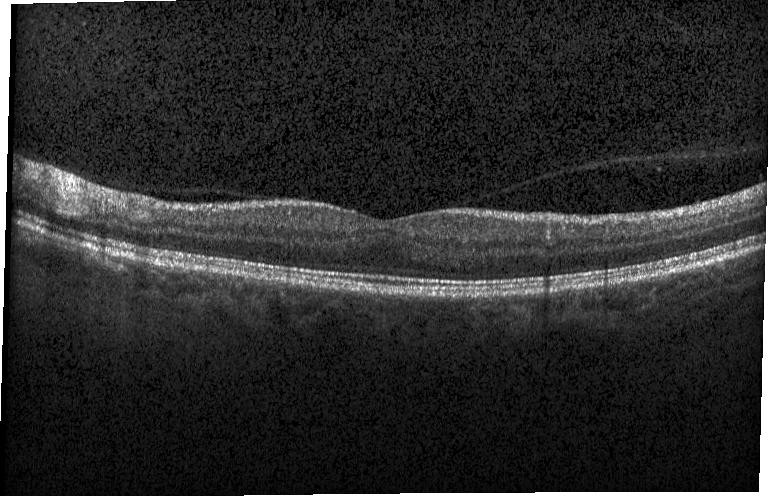 Retinal OCT cross-section, Heidelberg Spectralis OCT system, through the macula — Impression: no choroidal neovascularization, no diabetic macular edema, and no drusen.